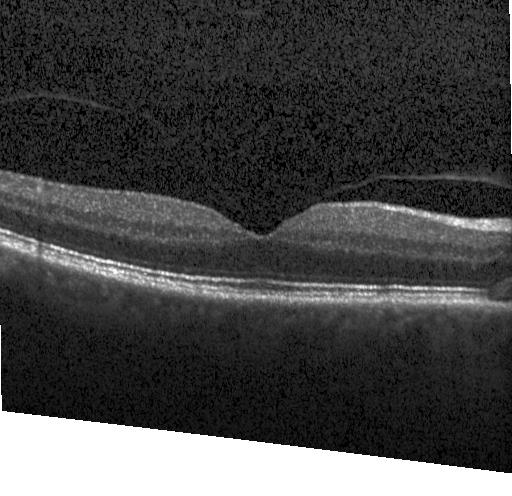
Diagnosis: no evidence of choroidal neovascularization, diabetic macular edema, or drusen.